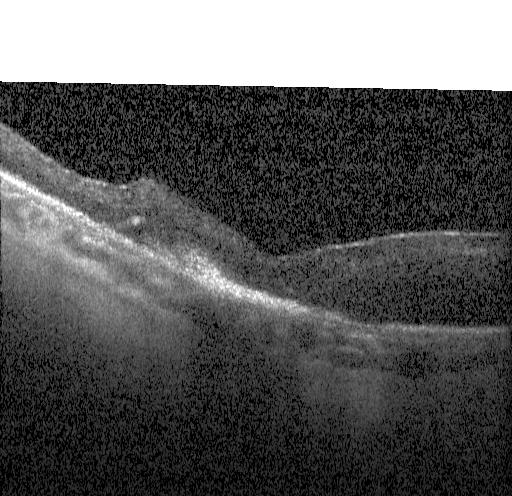 The scan shows choroidal neovascularization.